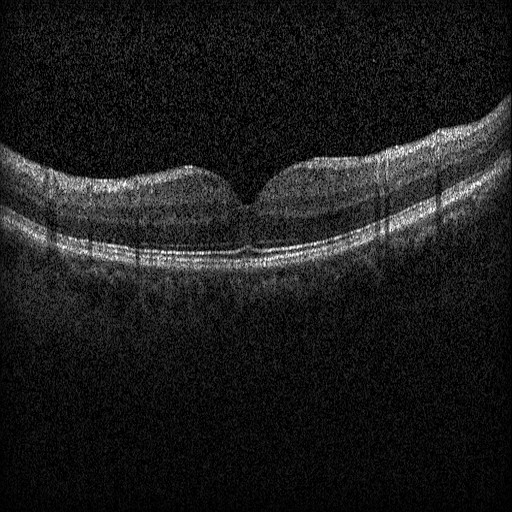
OCT finding: diabetic macular edema (DME).